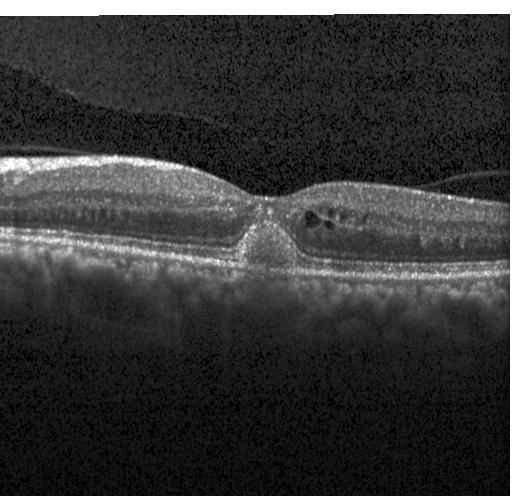 Macular OCT demonstrating CNV.